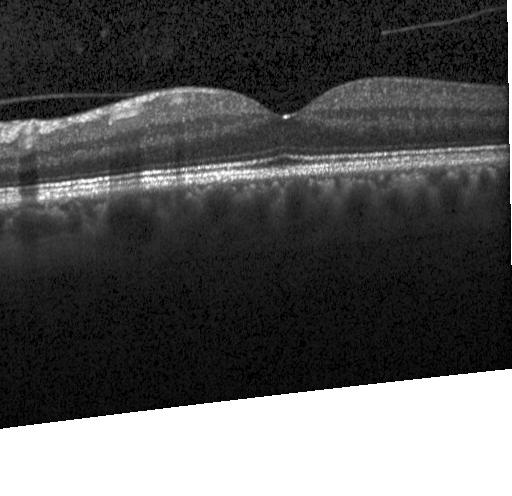 Impression: no evidence of choroidal neovascularization, diabetic macular edema, or drusen.